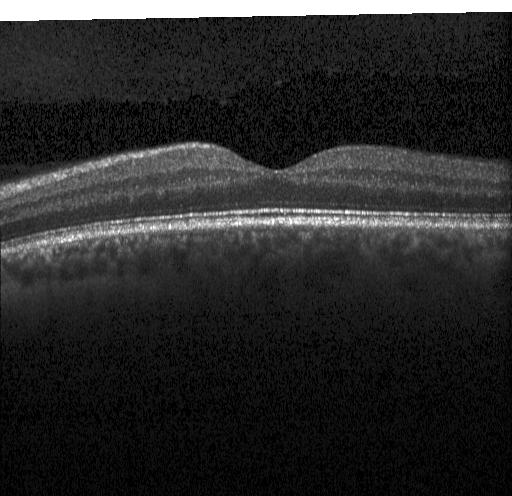

Optical coherence tomography scan, horizontal scan through the fovea. The scan shows no choroidal neovascularization, no diabetic macular edema, and no drusen.